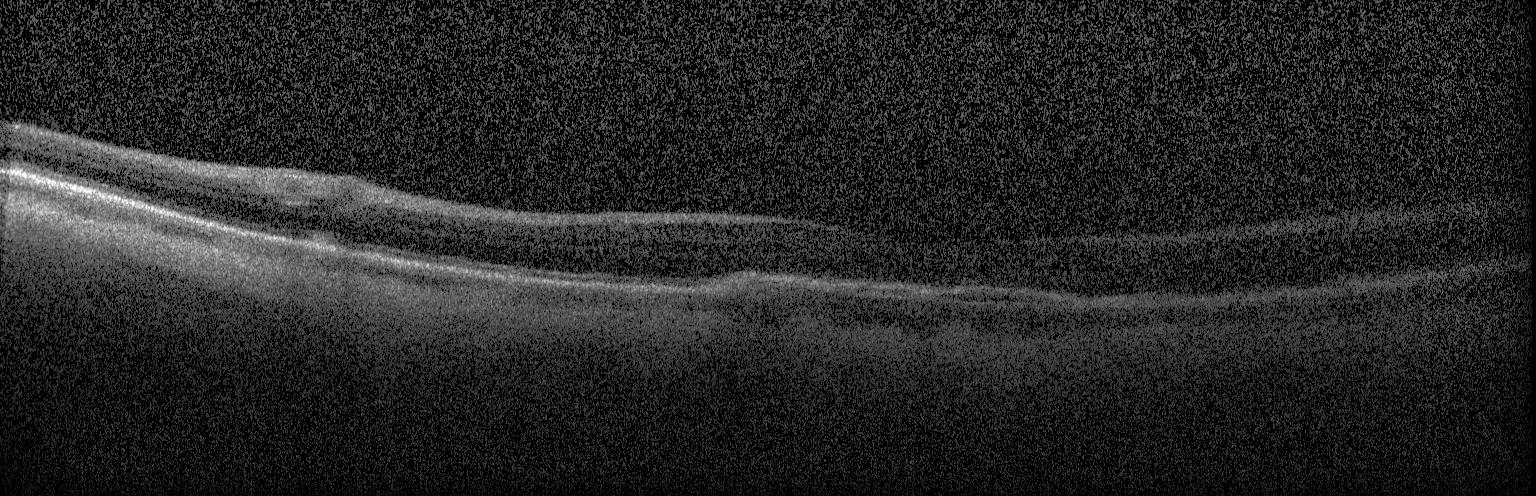
Diagnosis: choroidal neovascularization (CNV).